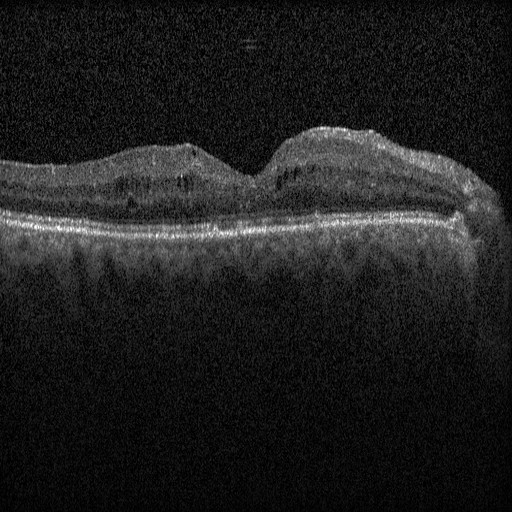
This B-scan demonstrates DME.